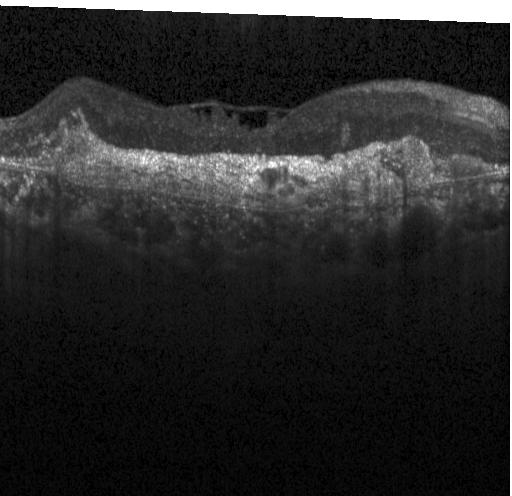 Optical coherence tomography scan. SD-OCT. Macular scan. Instrument: Heidelberg Spectralis — Assessment: a choroidal neovascular membrane.